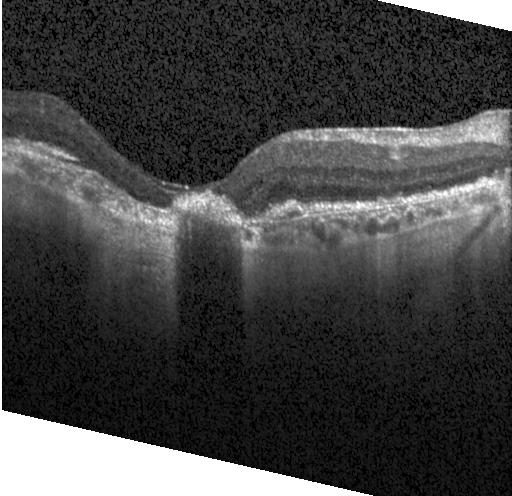

Retinal OCT cross-section showing choroidal neovascularization.